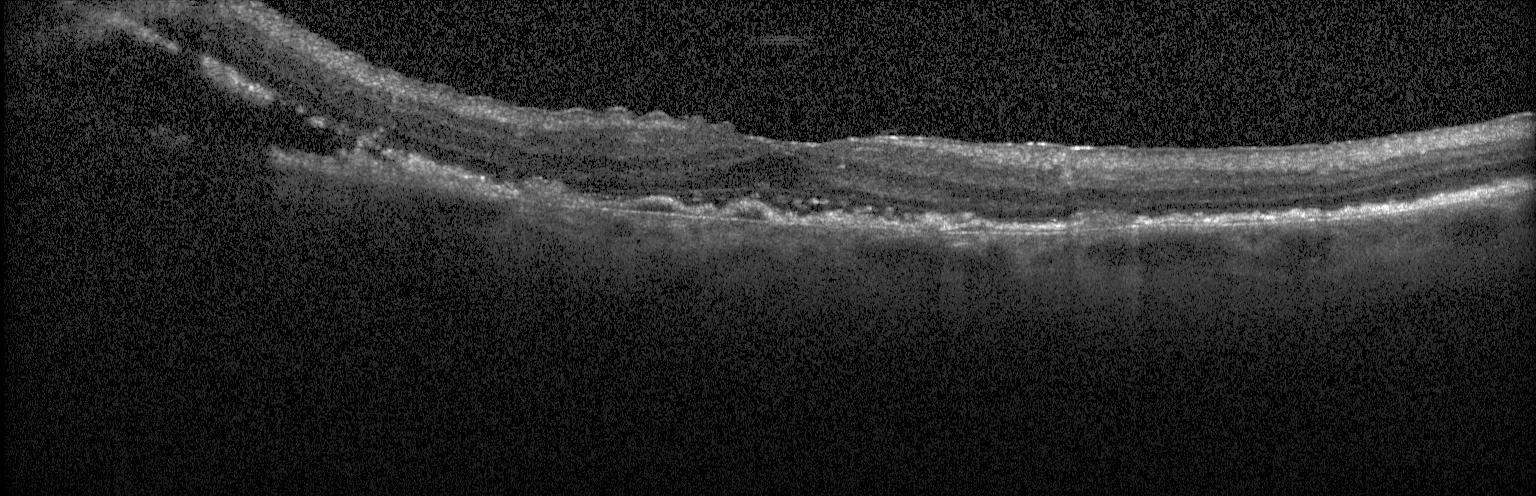
Retinal OCT B-scan. Macular scan — This B-scan demonstrates a choroidal neovascular membrane.